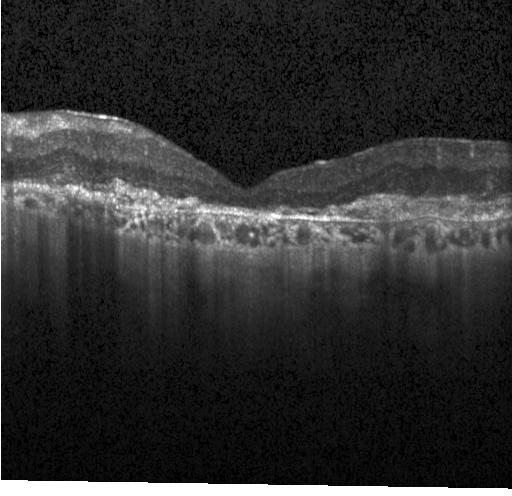
Horizontal scan through the fovea; spectral-domain OCT; retinal OCT cross-section. Assessment: a choroidal neovascular membrane.